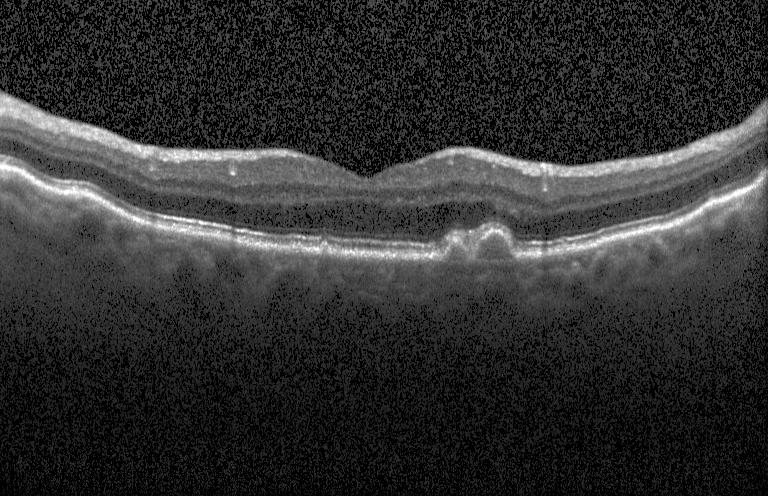
Retinal OCT B-scan.
Dx: drusen.